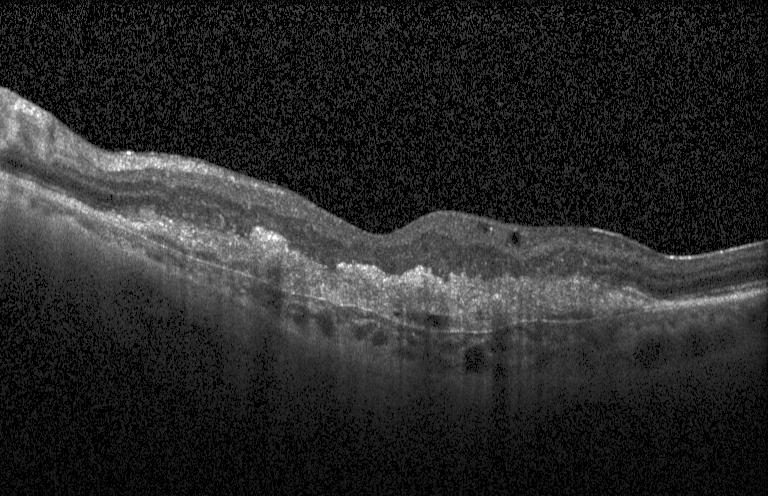
Impression: a choroidal neovascular membrane.